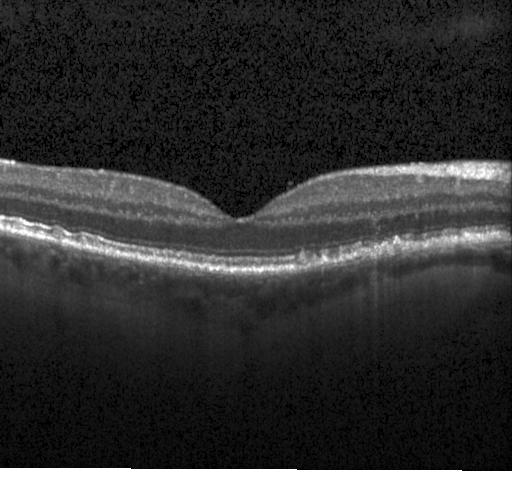

Optical coherence tomography B-scan, Heidelberg Spectralis OCT system, spectral-domain optical coherence tomography, fovea-centered — Sub-RPE drusenoid deposits.